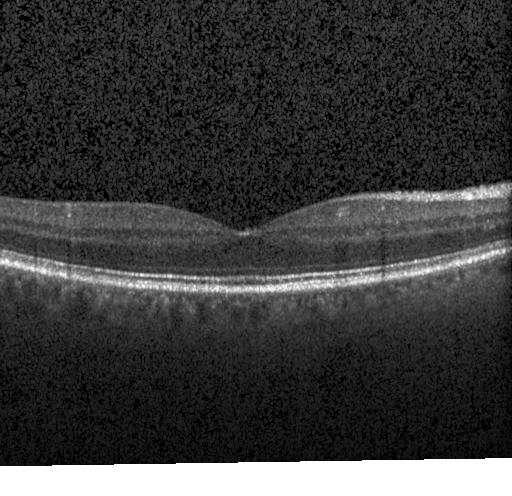 This B-scan demonstrates no CNV, no DME, and no drusen.